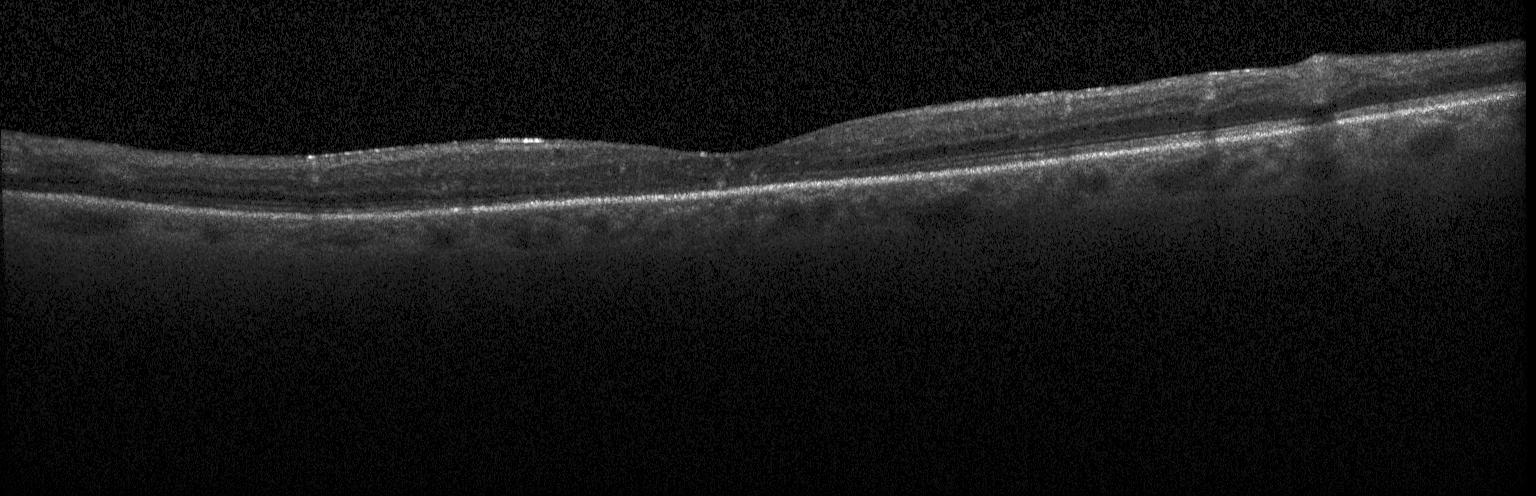 The scan shows no CNV, no DME, and no drusen.